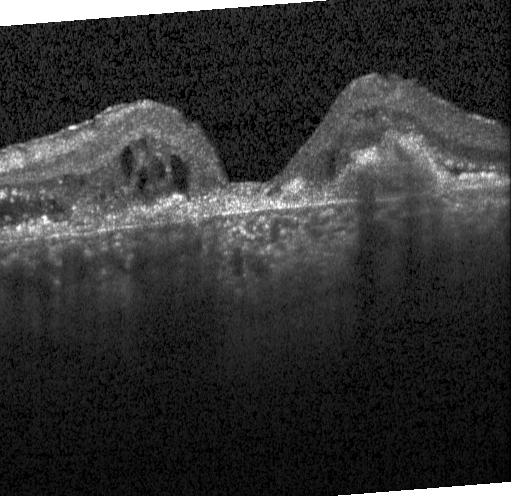
Finding: choroidal neovascularization.